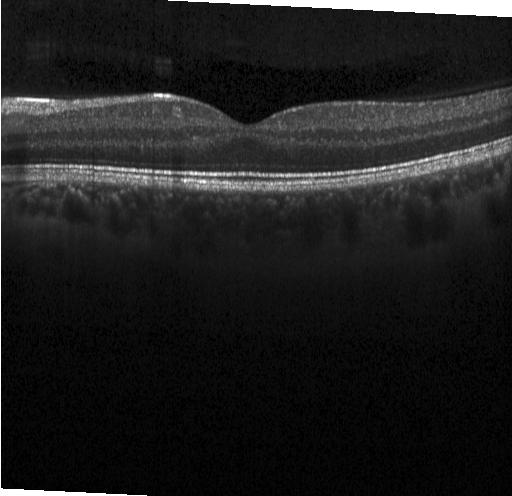
Optical coherence tomography scan
OCT finding: no choroidal neovascularization, no diabetic macular edema, and no drusen.